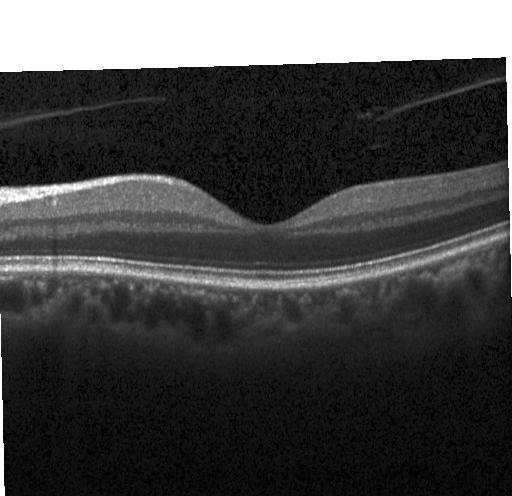
OCT line scan.
Finding: no choroidal neovascularization, no diabetic macular edema, and no drusen.